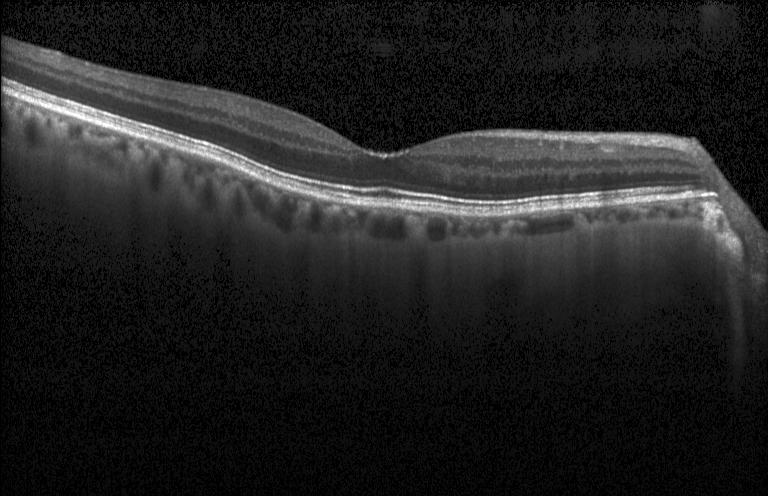

SD-OCT, retinal OCT B-scan — Assessment: neither CNV, DME, nor drusen.